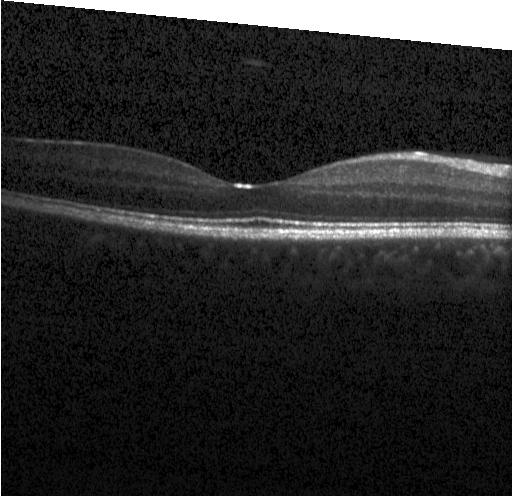 Retinal OCT cross-section · horizontal scan through the fovea · Heidelberg Spectralis. OCT finding: no choroidal neovascularization, diabetic macular edema, or drusen.